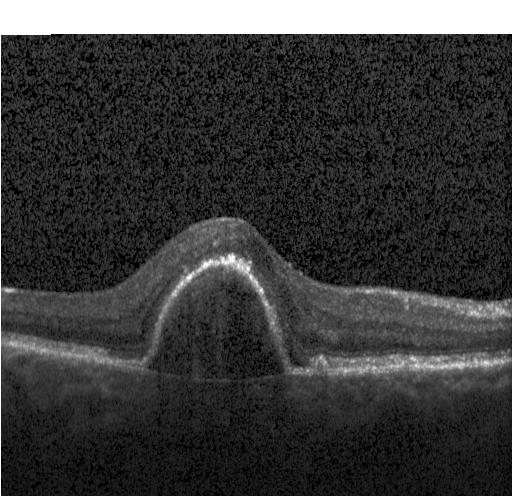
Spectral-domain OCT; centered on the fovea; retinal OCT B-scan; Heidelberg Spectralis.
Finding: a choroidal neovascular membrane.